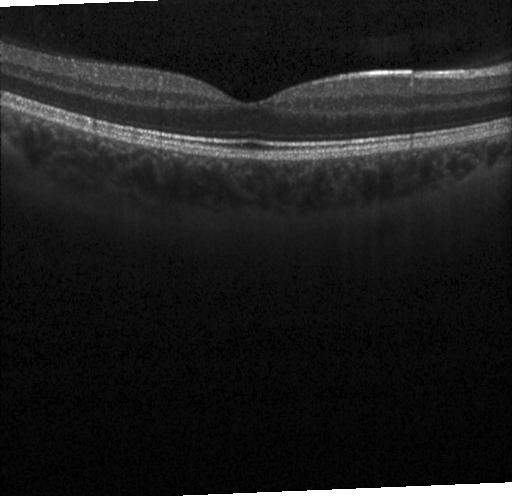
No choroidal neovascularization, diabetic macular edema, or drusen.